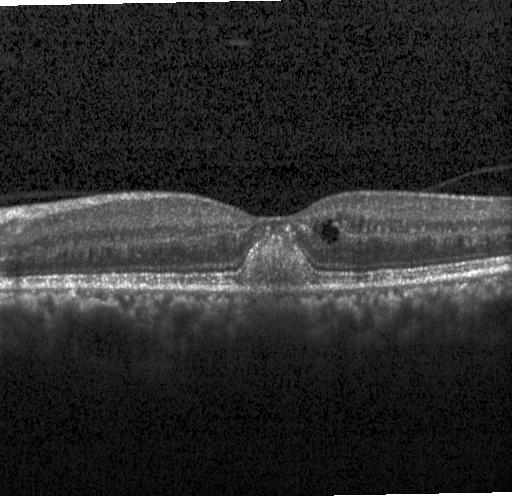
Fovea-centered, Heidelberg Spectralis OCT system, retinal OCT B-scan, spectral-domain OCT
Finding: CNV.